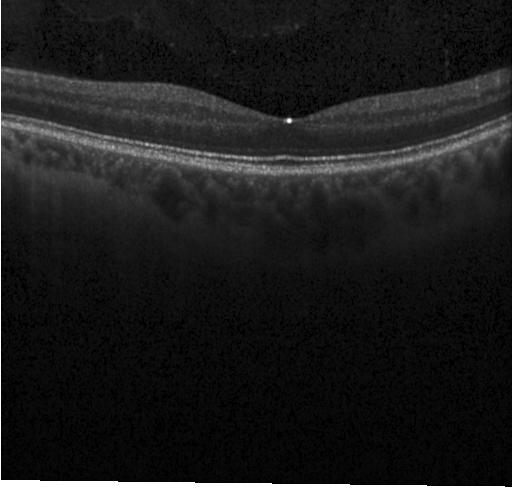
Optical coherence tomography scan. Impression: neither choroidal neovascularization, diabetic macular edema, nor drusen.